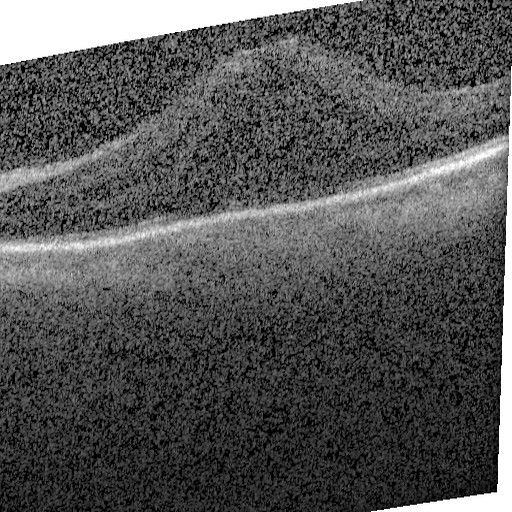

Finding: diabetic macular edema (DME).